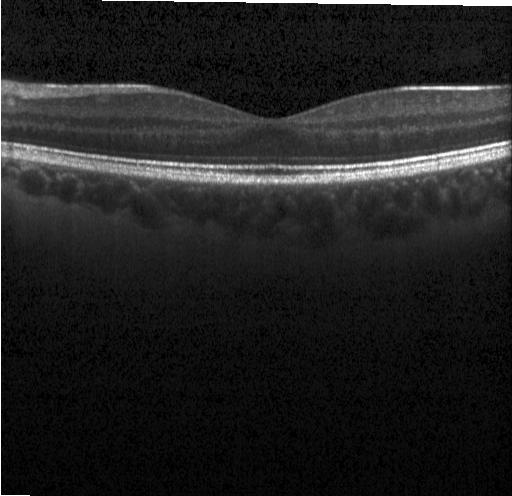

Acquired on a Heidelberg Spectralis. Retinal OCT cross-section. The scan shows no choroidal neovascularization, diabetic macular edema, or drusen.